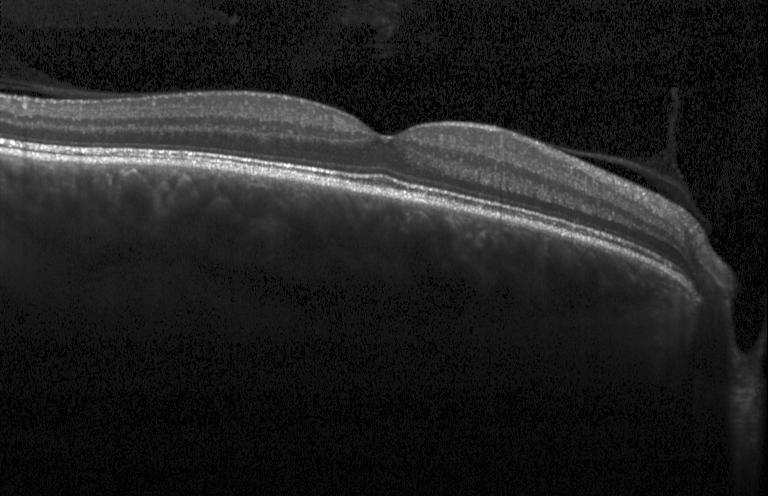 Optical coherence tomography B-scan — OCT finding: no choroidal neovascularization, diabetic macular edema, or drusen.